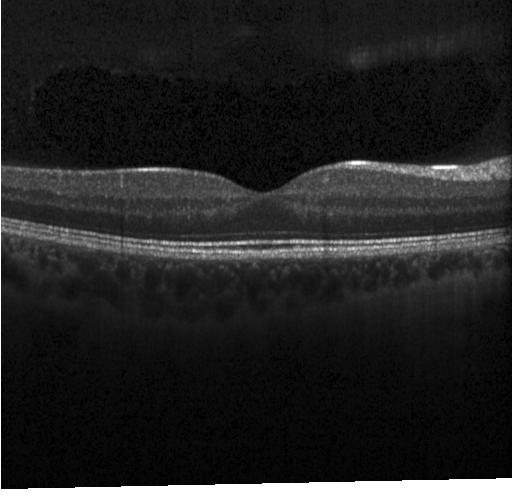 Finding: no choroidal neovascularization, diabetic macular edema, or drusen.